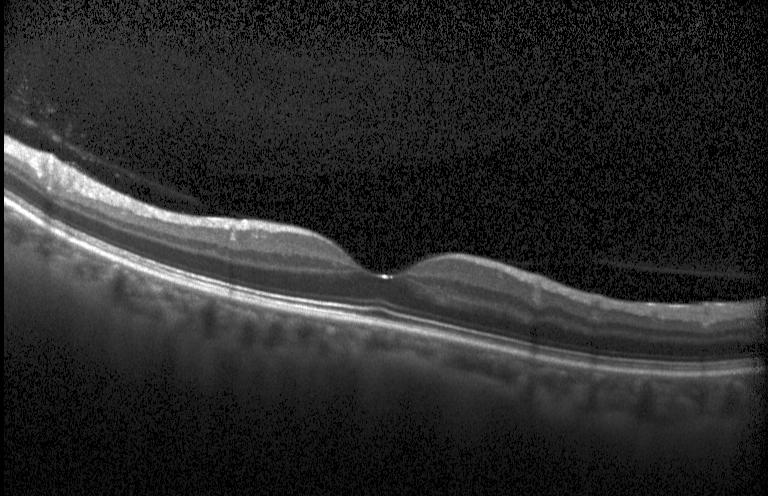 Centered on the fovea, optical coherence tomography B-scan.
Diagnosis: no CNV, DME, or drusen.